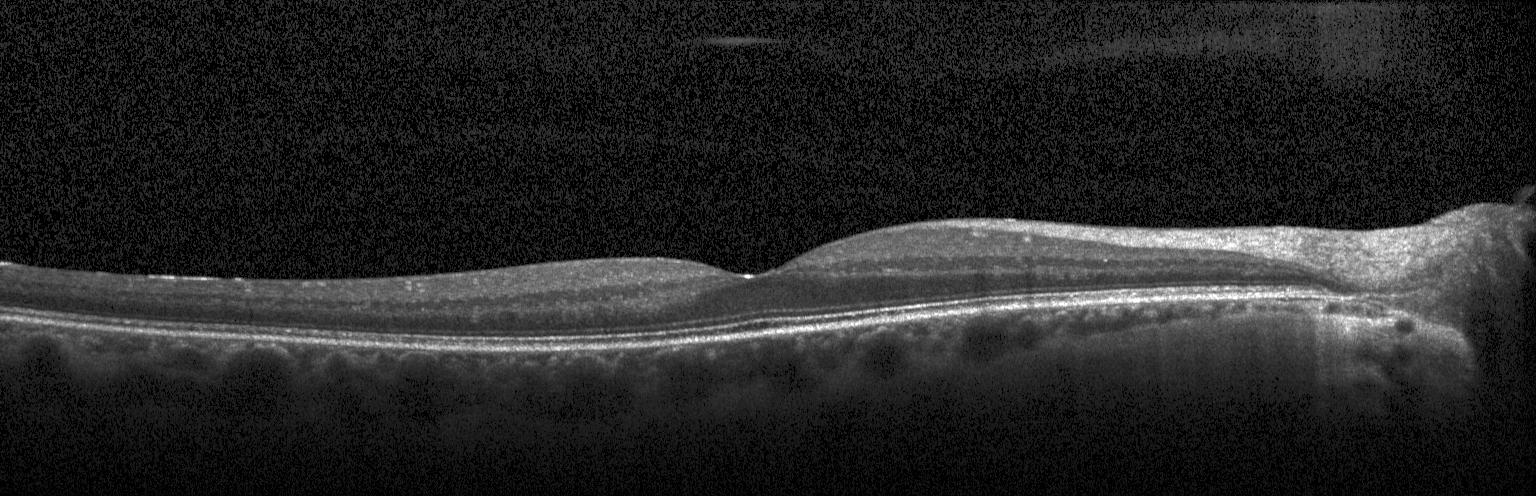
Centered on the fovea · spectral-domain optical coherence tomography · optical coherence tomography scan · instrument: Heidelberg Spectralis. This B-scan demonstrates no choroidal neovascularization, no diabetic macular edema, and no drusen.